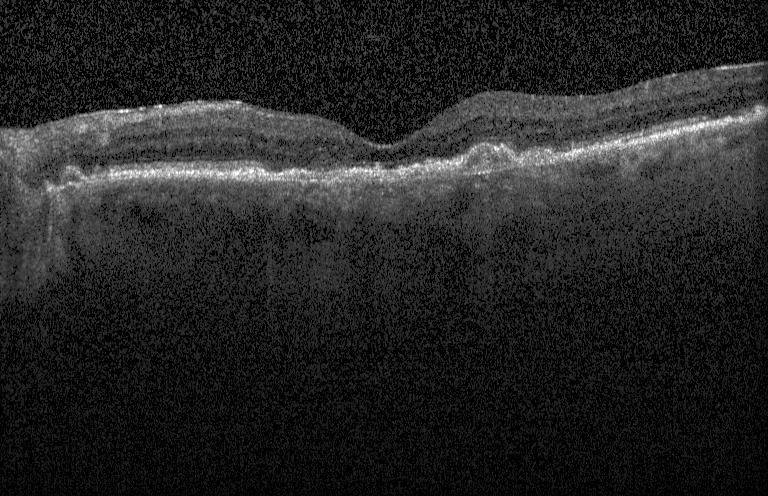
SD-OCT. Optical coherence tomography B-scan. Heidelberg Spectralis. Horizontal scan through the fovea
Assessment: CNV.